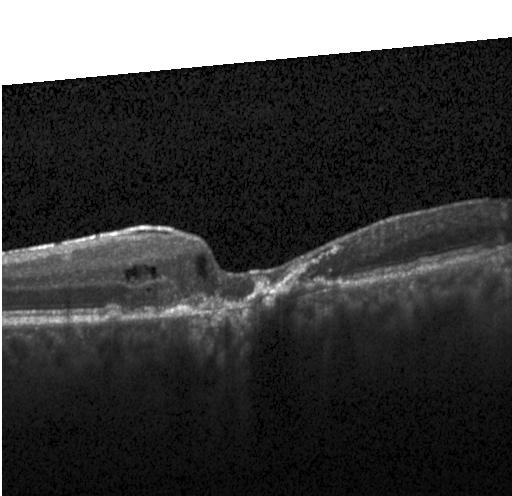
Finding: CNV.